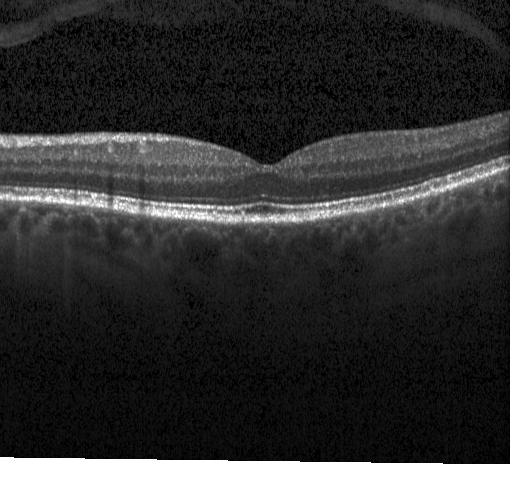 Retinal OCT B-scan — Diagnosis: no evidence of choroidal neovascularization, diabetic macular edema, or drusen.